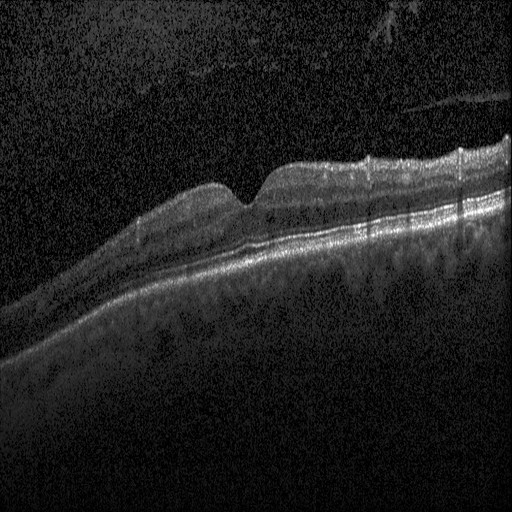

Impression: diabetic macular edema (DME).